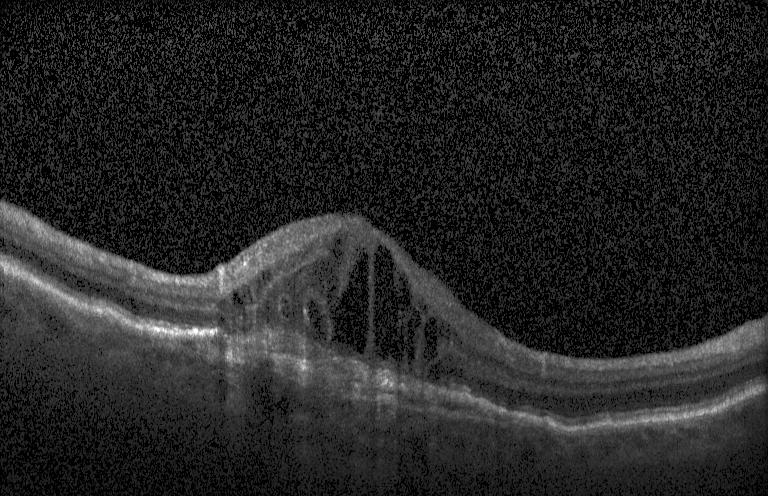 Centered on the fovea. Retinal OCT cross-section. Acquired on a Heidelberg Spectralis. Spectral-domain optical coherence tomography.
Choroidal neovascularization.